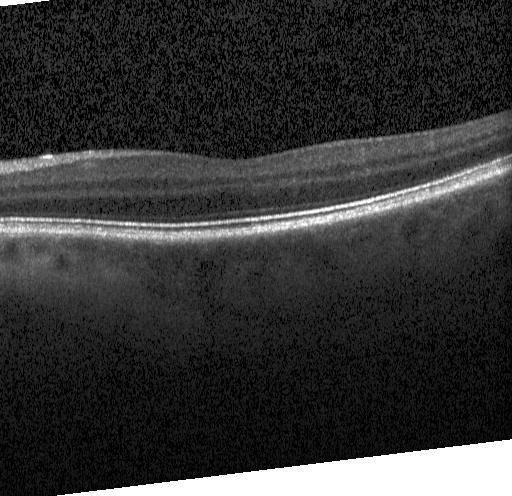
Finding: no choroidal neovascularization, no diabetic macular edema, and no drusen.